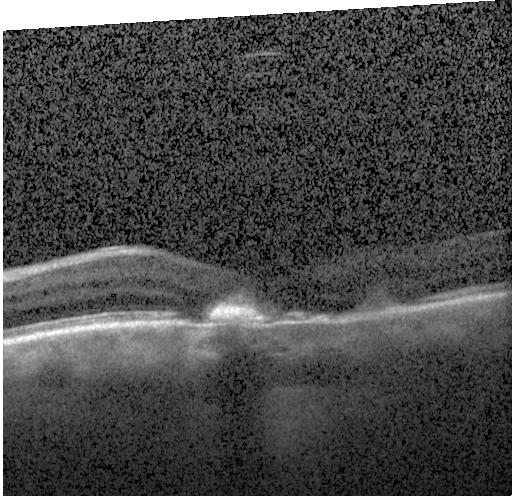

Dx: a choroidal neovascular membrane.